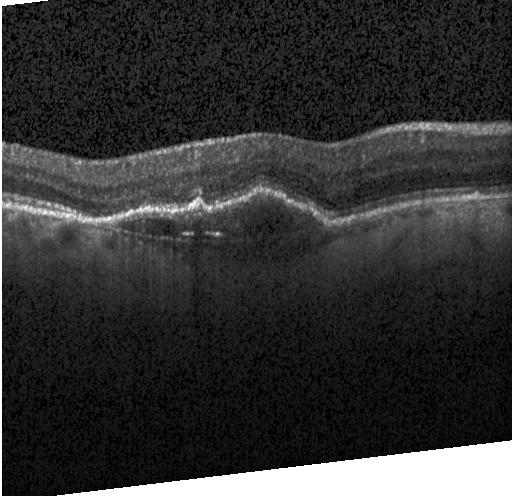
Finding: CNV.